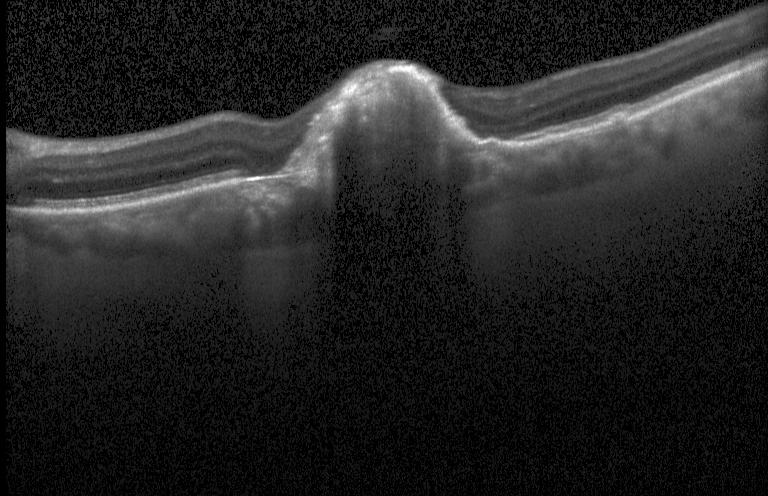

Through the macula; OCT B-scan
Impression: choroidal neovascularization (CNV).